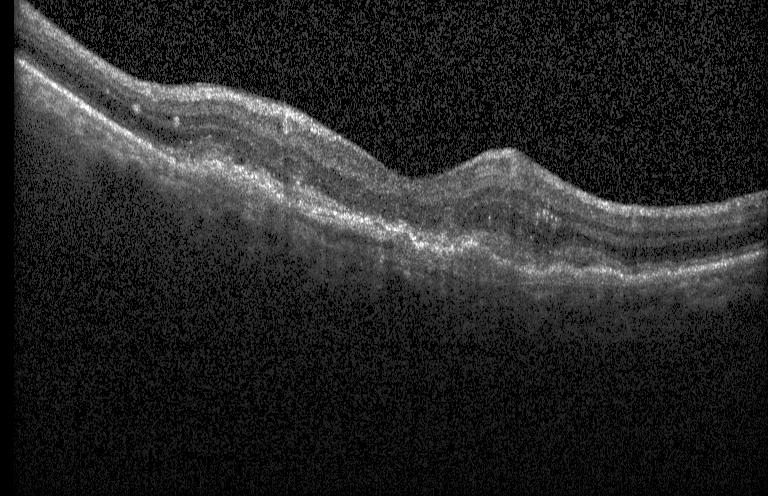 Centered on the fovea · acquired on a Heidelberg Spectralis · retinal OCT B-scan. CNV.